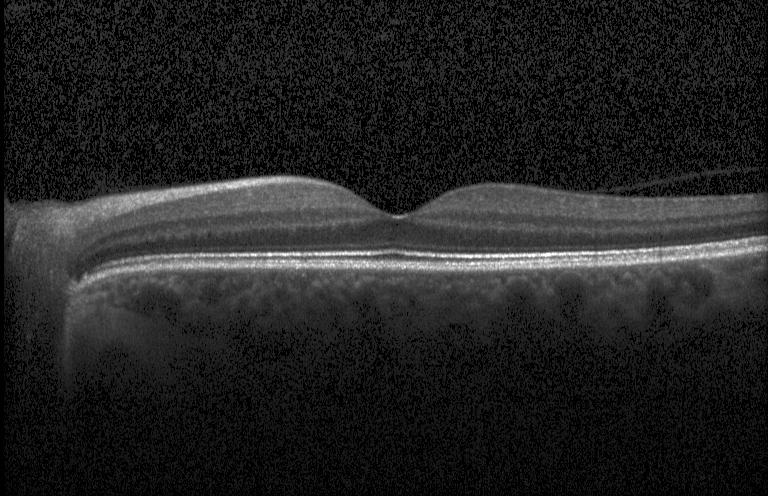 Impression: no choroidal neovascularization, no diabetic macular edema, and no drusen.